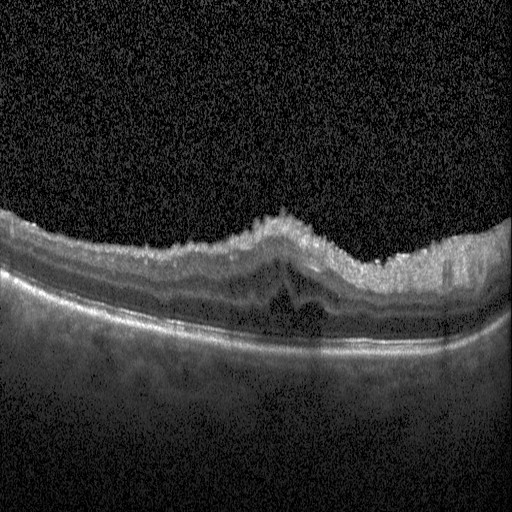 Optical coherence tomography B-scan, Heidelberg Spectralis OCT system, macular scan, SD-OCT
Finding: diabetic macular edema (DME).